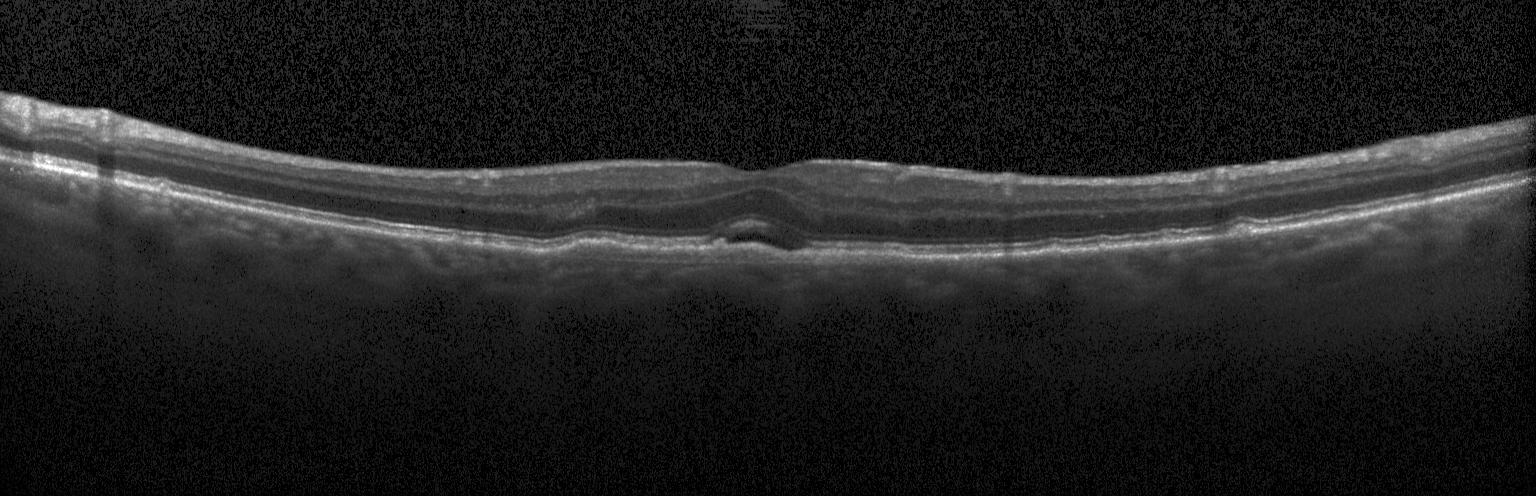 Optical coherence tomography B-scan. Acquired on a Heidelberg Spectralis
This B-scan demonstrates a choroidal neovascular membrane.